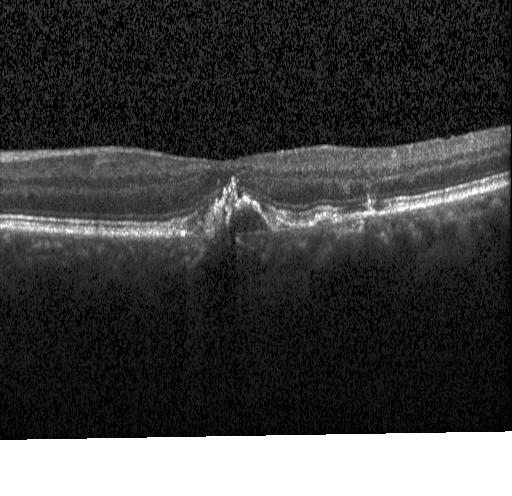 OCT scan showing a choroidal neovascular membrane.